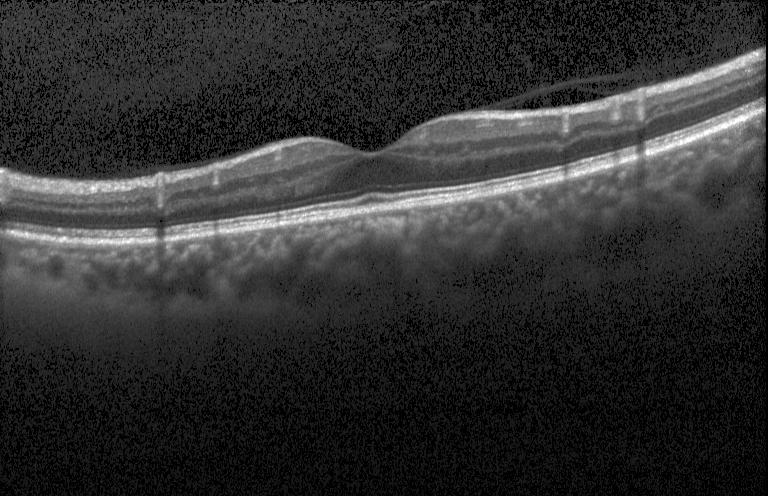

OCT finding: no evidence of CNV, DME, or drusen.